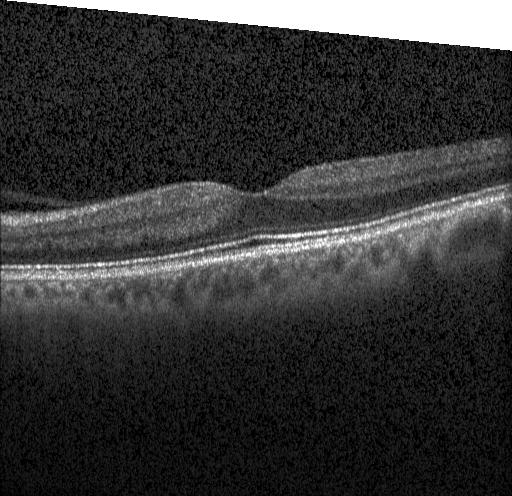

Optical coherence tomography scan — This B-scan demonstrates no choroidal neovascularization, diabetic macular edema, or drusen.